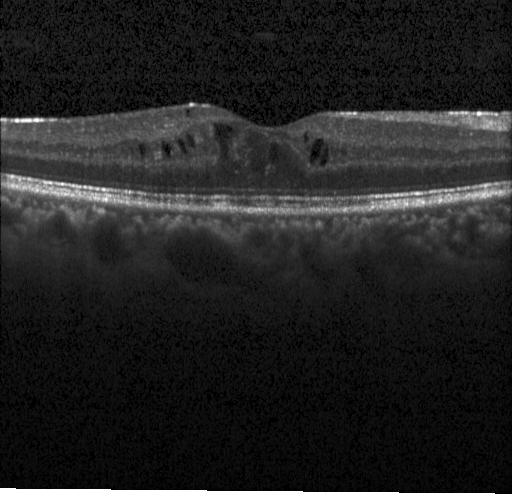

Diabetic macular edema.